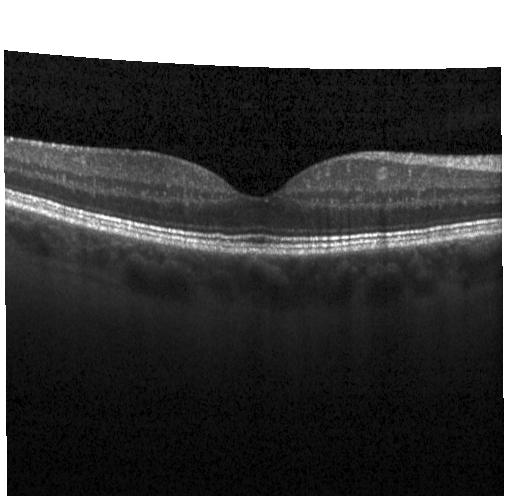 Macular OCT: neither choroidal neovascularization, diabetic macular edema, nor drusen.